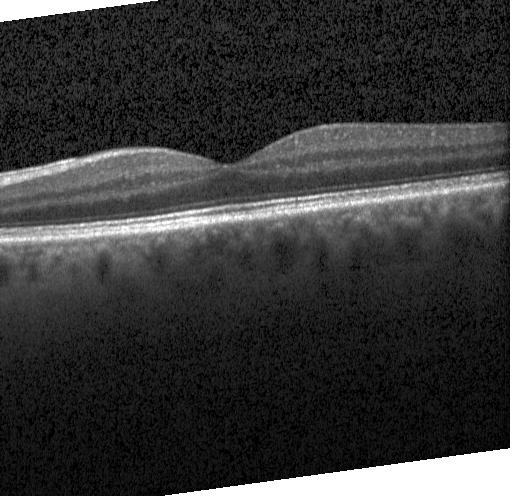 Retinal OCT cross-section; Heidelberg Spectralis; spectral-domain OCT — Impression: no choroidal neovascularization, diabetic macular edema, or drusen.